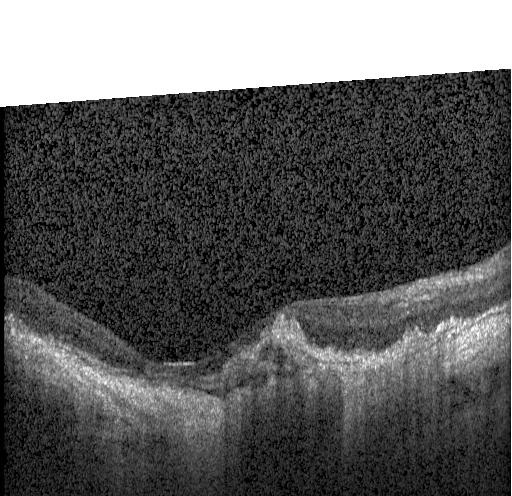 Optical coherence tomography scan · spectral-domain optical coherence tomography · Heidelberg Spectralis
The scan shows CNV.